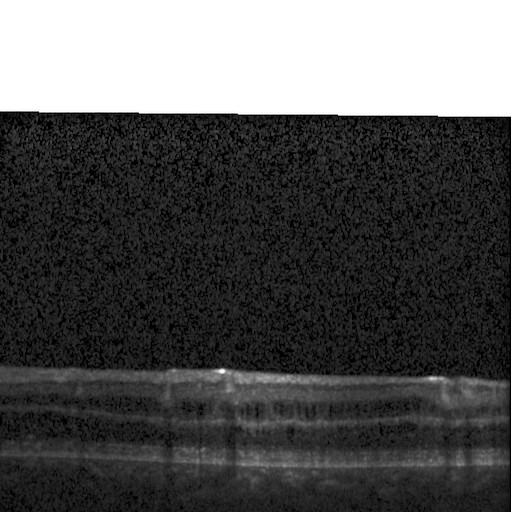
Instrument: Heidelberg Spectralis, SD-OCT, OCT B-scan
Dx: diabetic macular edema.